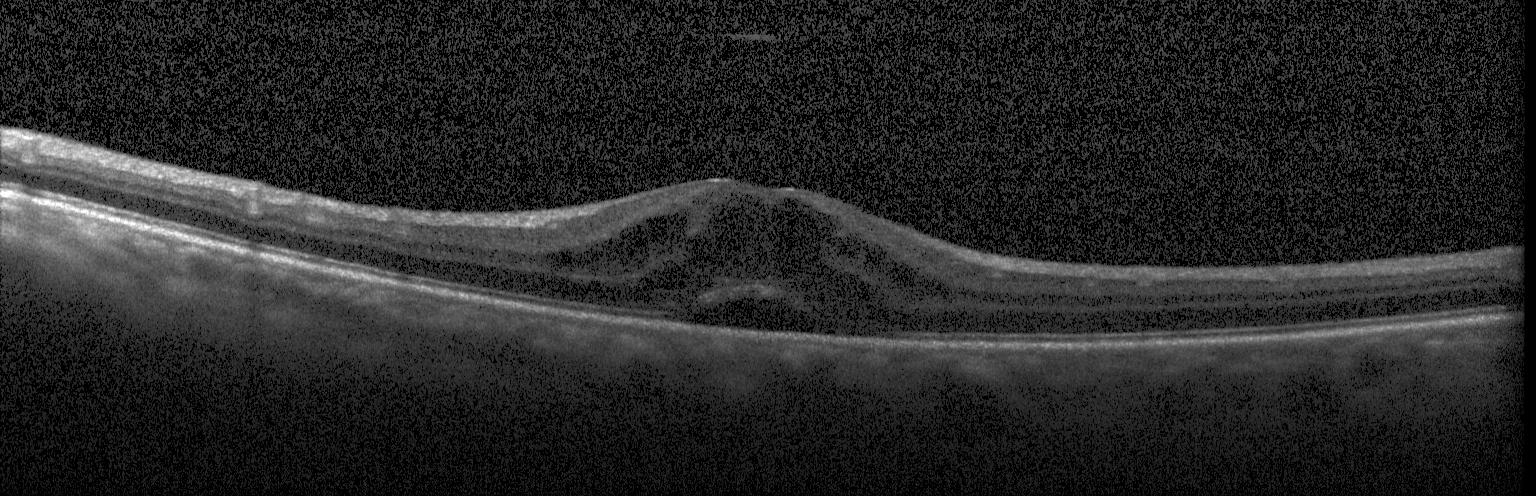 Heidelberg Spectralis · macular scan · SD-OCT · optical coherence tomography B-scan. DME.